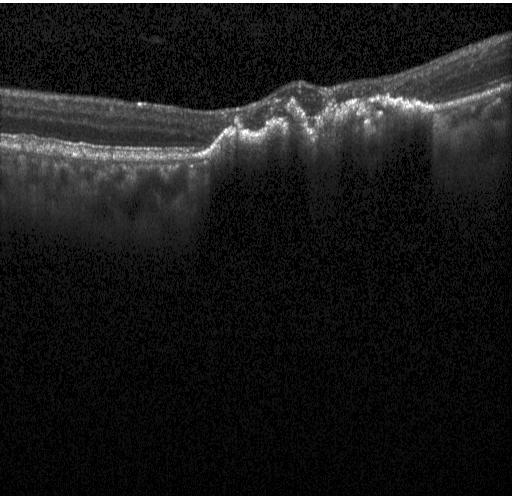

The scan shows choroidal neovascularization (CNV).